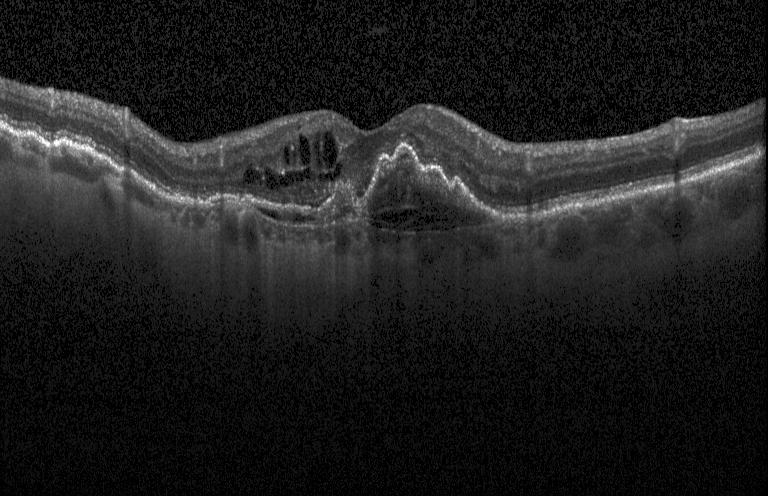
This B-scan demonstrates a choroidal neovascular membrane.